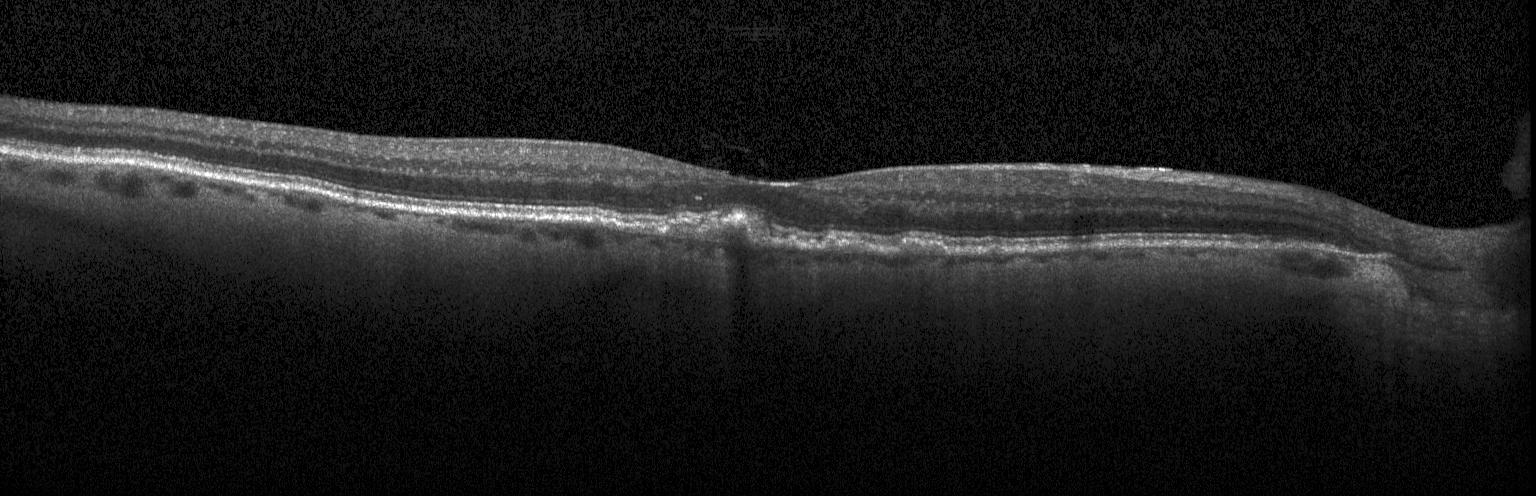
Retinal OCT B-scan · instrument: Heidelberg Spectralis · through the macula.
Diagnosis: multiple drusen.